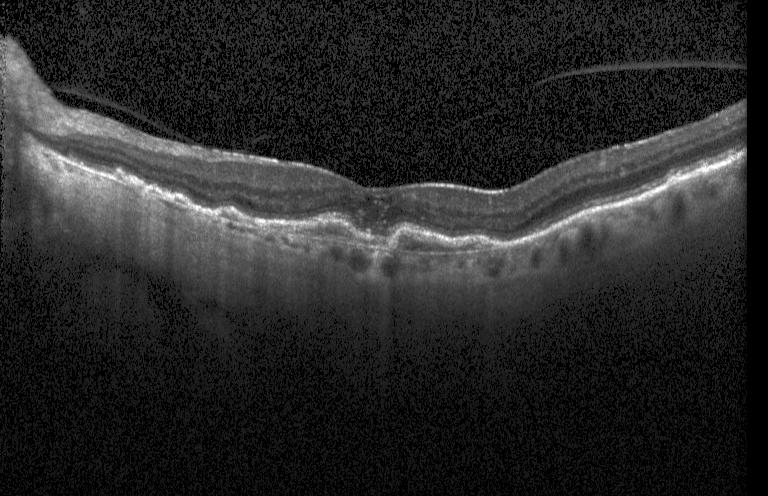
Fovea-centered · optical coherence tomography B-scan — Dx: a choroidal neovascular membrane.